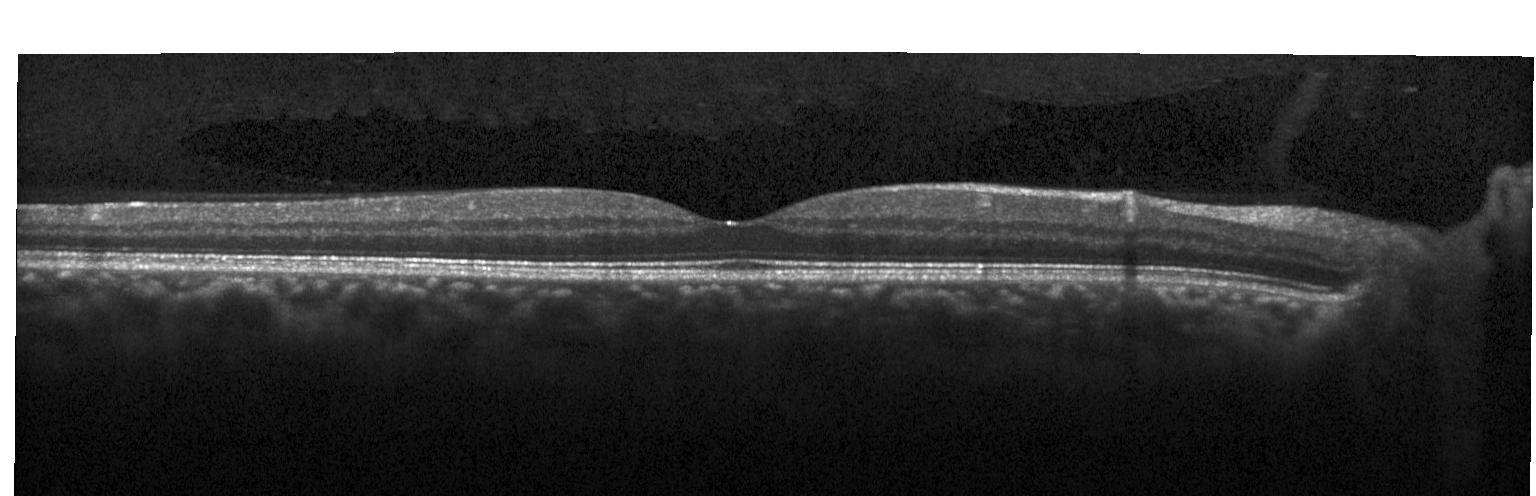 Optical coherence tomography scan — No evidence of choroidal neovascularization, diabetic macular edema, or drusen.